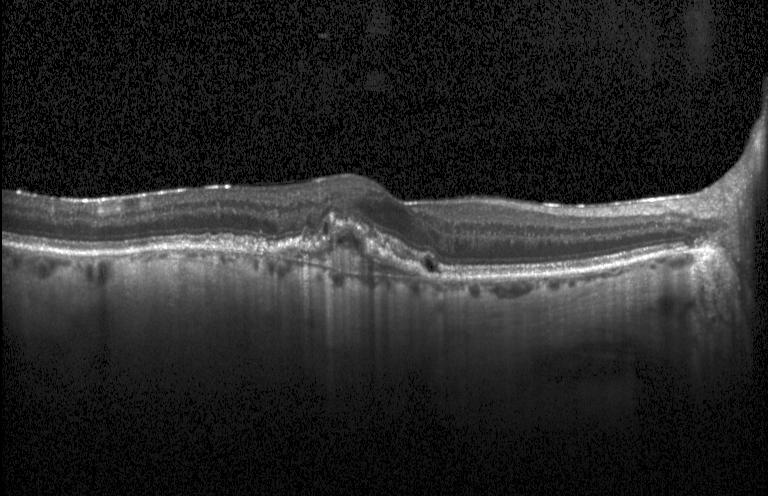

Impression: a choroidal neovascular membrane.